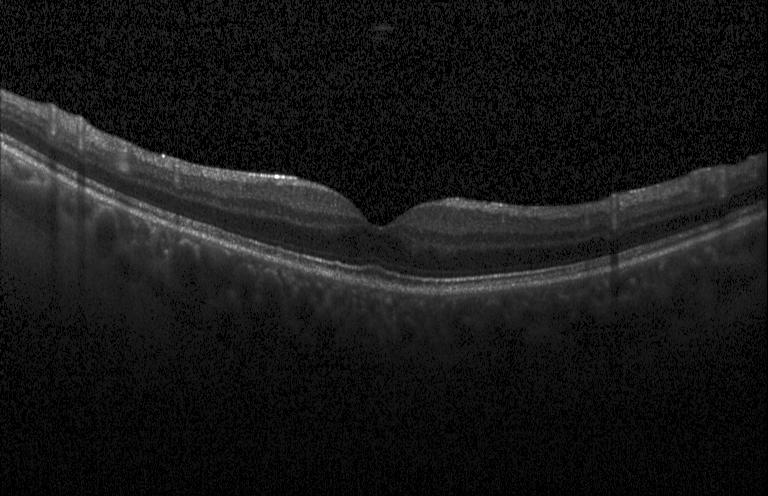

Impression: no choroidal neovascularization, no diabetic macular edema, and no drusen.